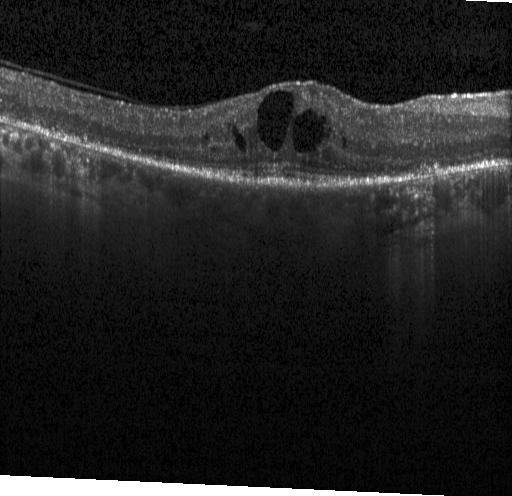

Assessment: diabetic macular edema.